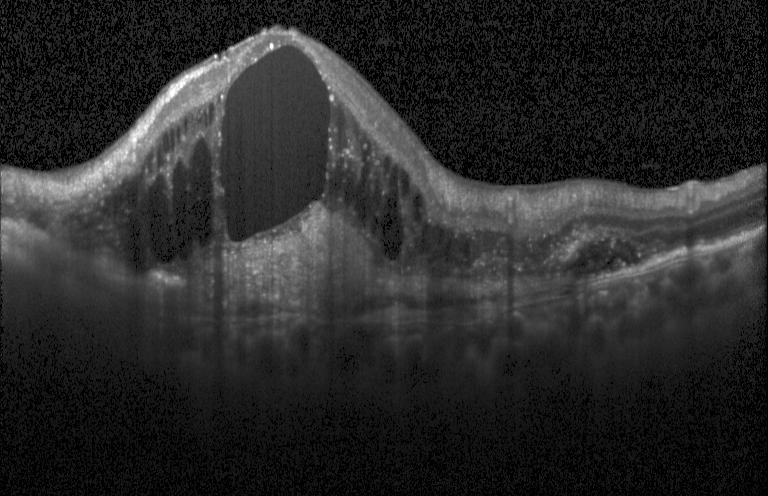
Macular scan. Spectral-domain optical coherence tomography. Optical coherence tomography scan — Diagnosis: diabetic macular edema.